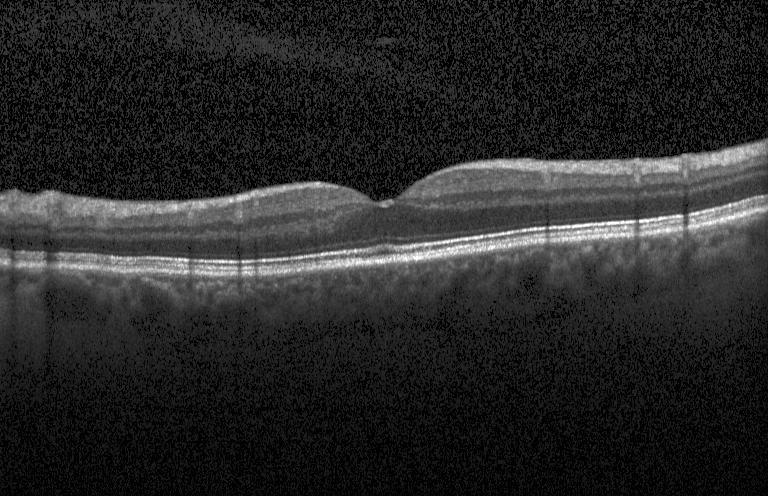
OCT line scan, SD-OCT. This B-scan demonstrates no choroidal neovascularization, no diabetic macular edema, and no drusen.